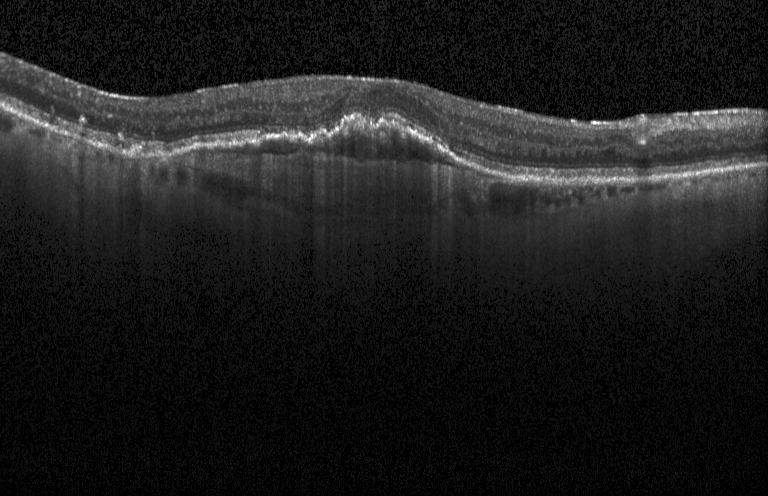

Assessment: CNV.